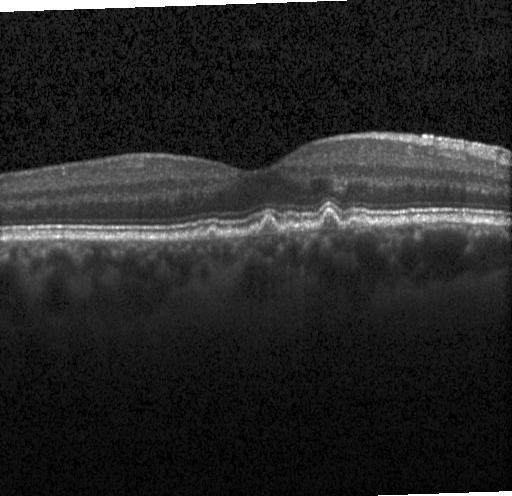

Macular scan. Acquired on a Heidelberg Spectralis. Spectral-domain OCT. Optical coherence tomography B-scan. Finding: drusen.